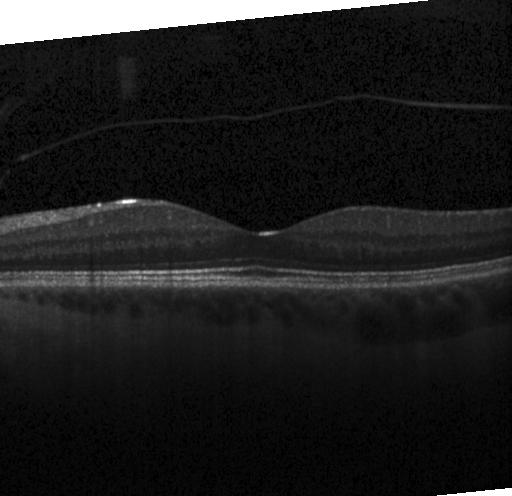 OCT finding: no choroidal neovascularization, no diabetic macular edema, and no drusen.